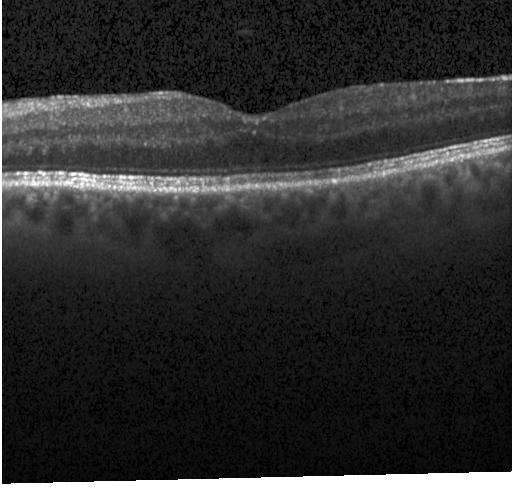
Macular scan · instrument: Heidelberg Spectralis · retinal OCT cross-section · spectral-domain OCT.
Finding: no choroidal neovascularization, diabetic macular edema, or drusen.